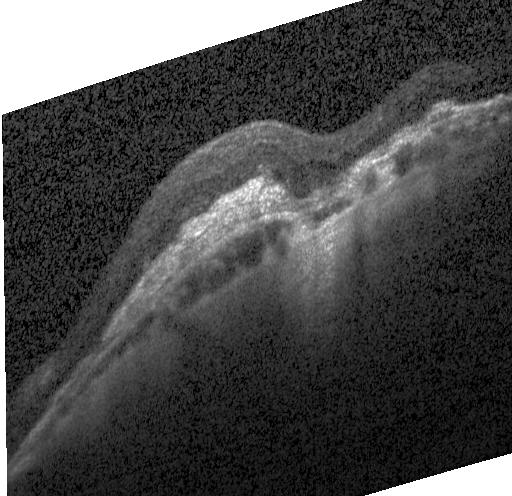

SD-OCT; centered on the fovea; optical coherence tomography scan
Macular OCT: choroidal neovascularization.